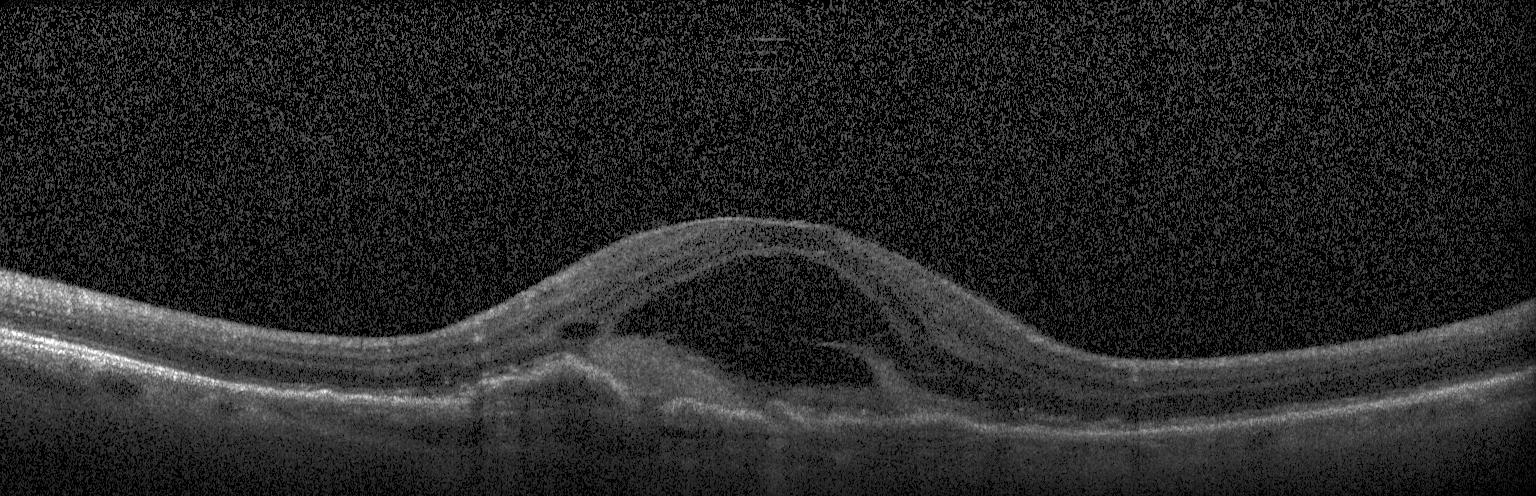
Finding: choroidal neovascularization (CNV).